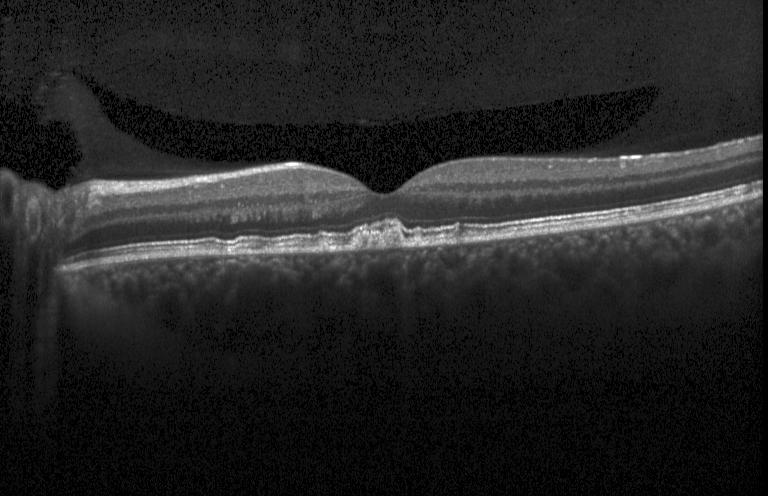

Diagnosis: drusen.